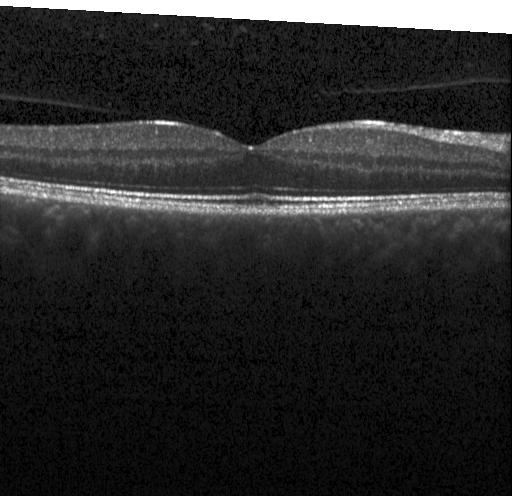

Dx: neither choroidal neovascularization, diabetic macular edema, nor drusen.